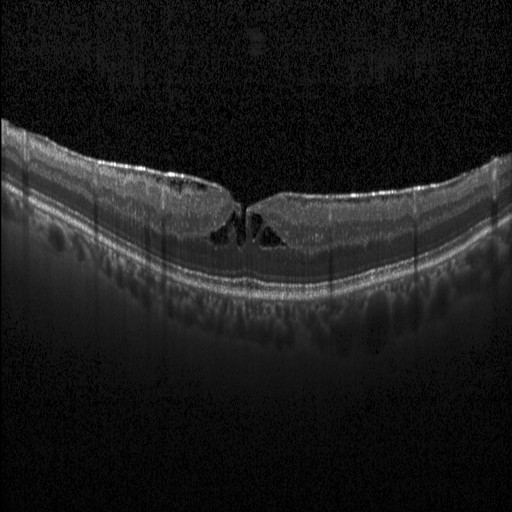
Spectral-domain OCT B-scan: diabetic macular edema (DME).